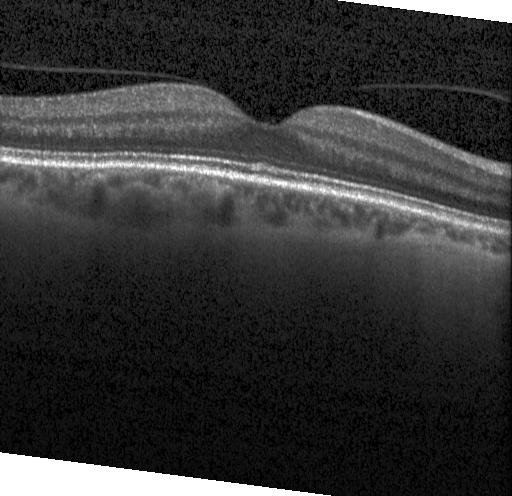
OCT line scan
Assessment: no CNV, DME, or drusen.